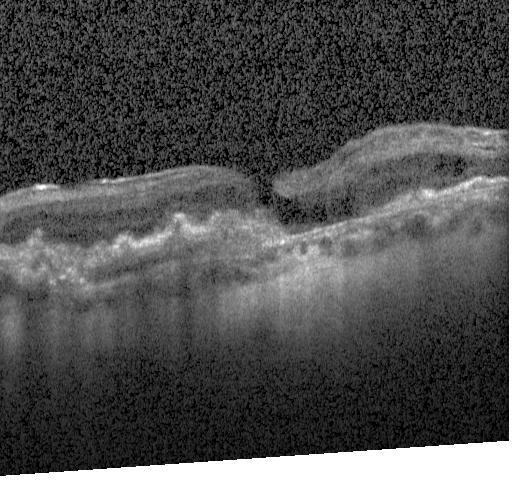 This B-scan demonstrates choroidal neovascularization (CNV).